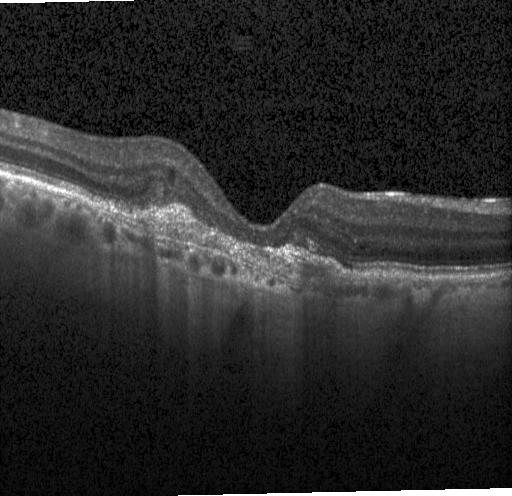

Spectral-domain OCT, optical coherence tomography B-scan, acquired on a Heidelberg Spectralis, through the macula
Assessment: a choroidal neovascular membrane.